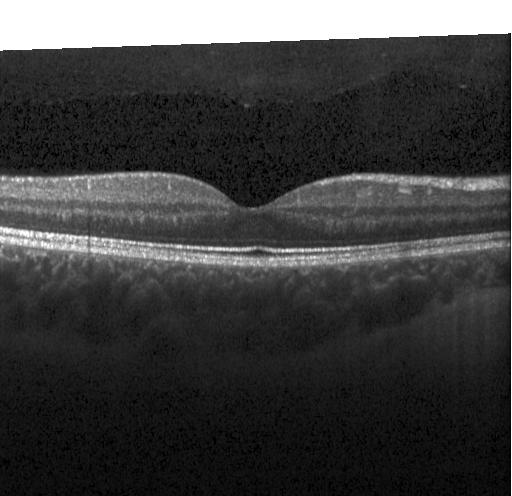 This B-scan demonstrates no choroidal neovascularization, no diabetic macular edema, and no drusen.